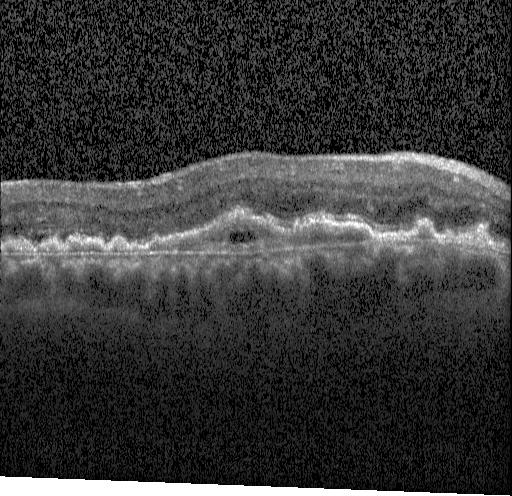

The scan shows CNV.